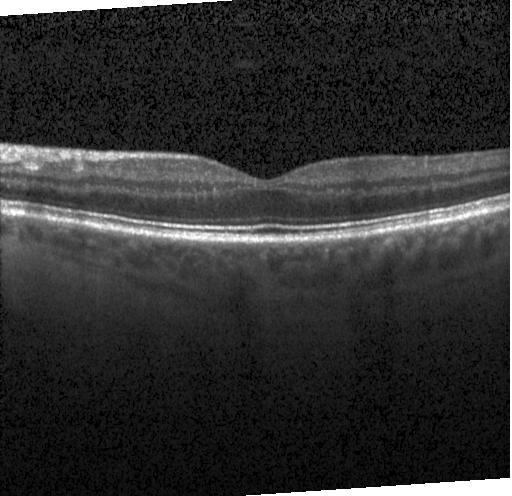 OCT B-scan showing no choroidal neovascularization, diabetic macular edema, or drusen.